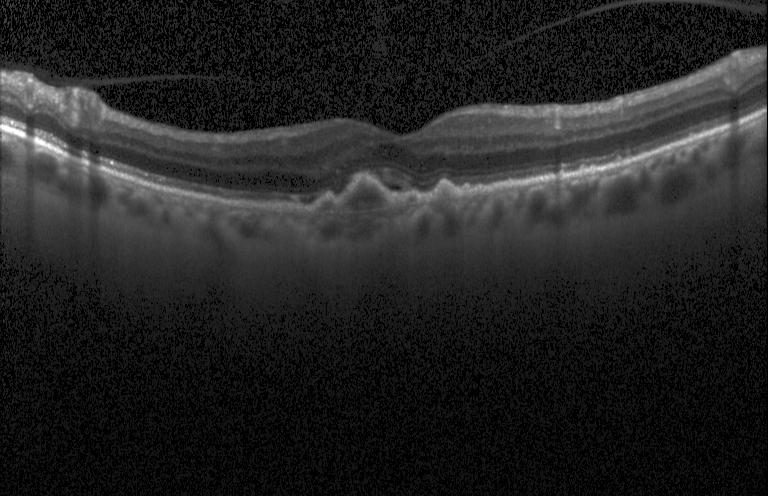
Diagnosis: choroidal neovascularization (CNV).